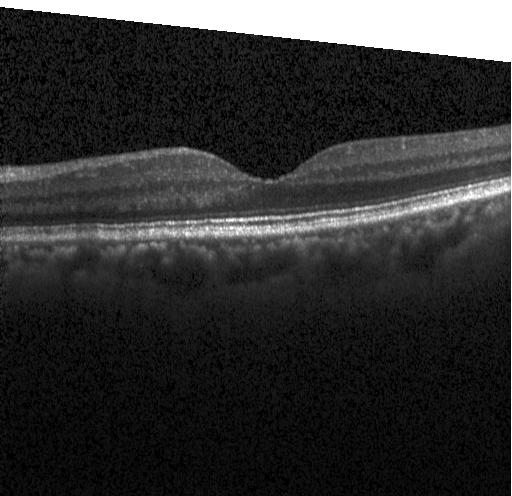
Instrument: Heidelberg Spectralis; horizontal scan through the fovea; retinal OCT B-scan
Finding: no CNV, DME, or drusen.